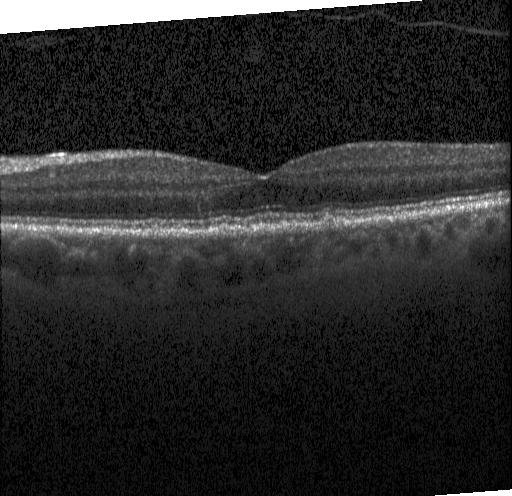 SD-OCT; horizontal scan through the fovea; retinal OCT B-scan; instrument: Heidelberg Spectralis
Macular OCT: drusen.